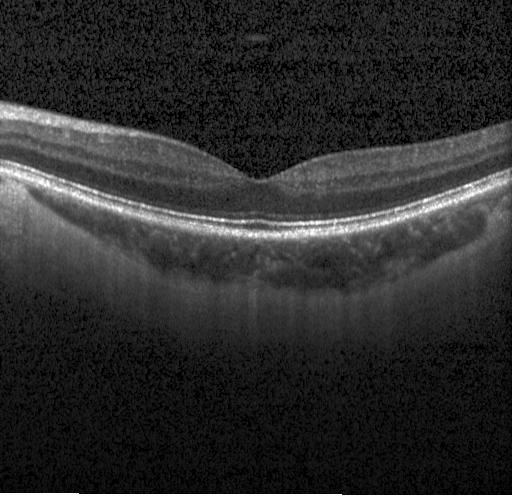

Retinal OCT B-scan
The scan shows neither choroidal neovascularization, diabetic macular edema, nor drusen.